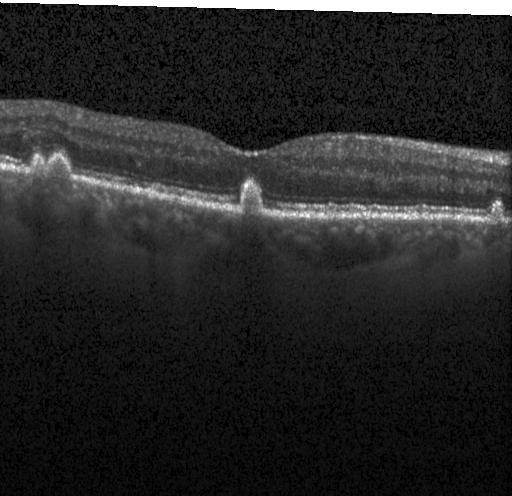
Finding: sub-RPE drusenoid deposits.